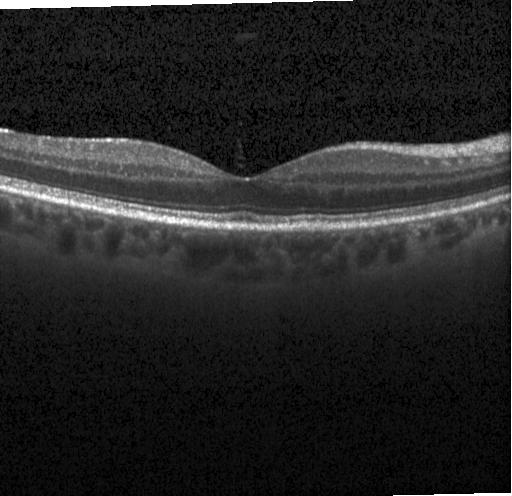

The scan shows neither choroidal neovascularization, diabetic macular edema, nor drusen.